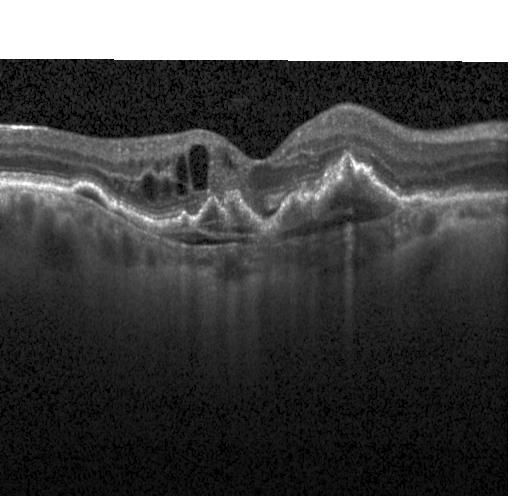
Spectral-domain OCT · instrument: Heidelberg Spectralis · OCT B-scan · through the macula — Assessment: choroidal neovascularization.